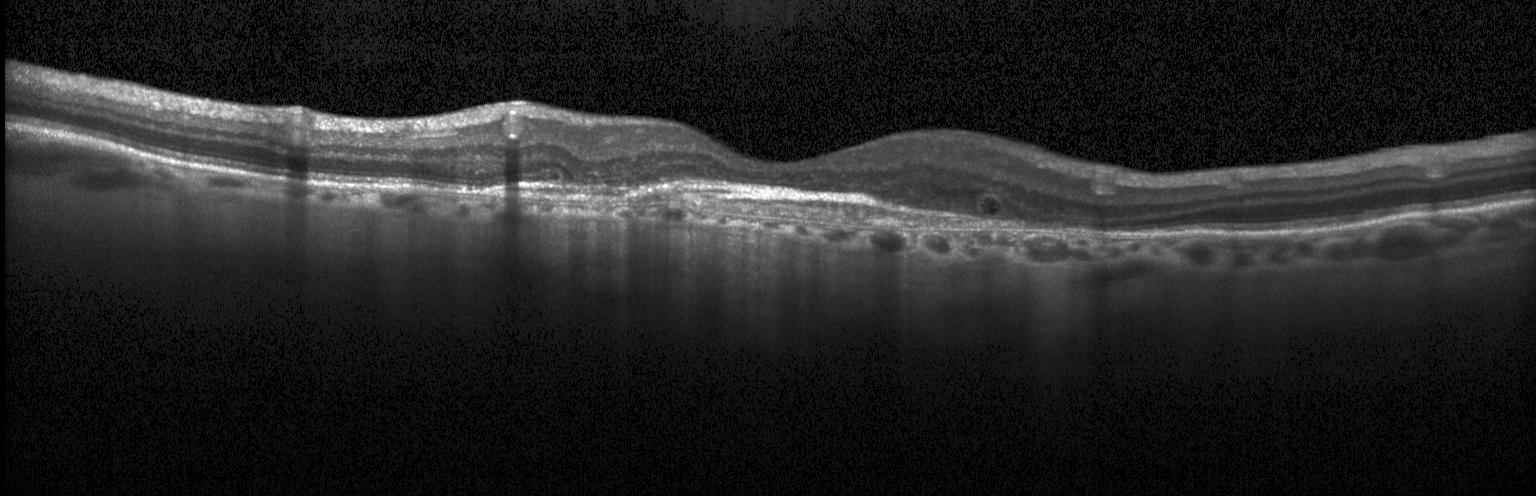

Retinal OCT cross-section showing a choroidal neovascular membrane.